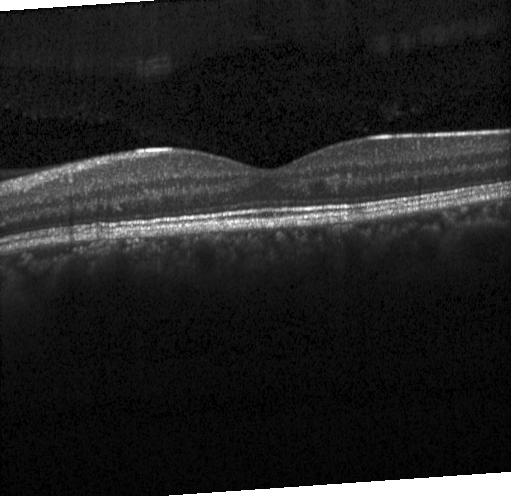 Assessment: neither choroidal neovascularization, diabetic macular edema, nor drusen.